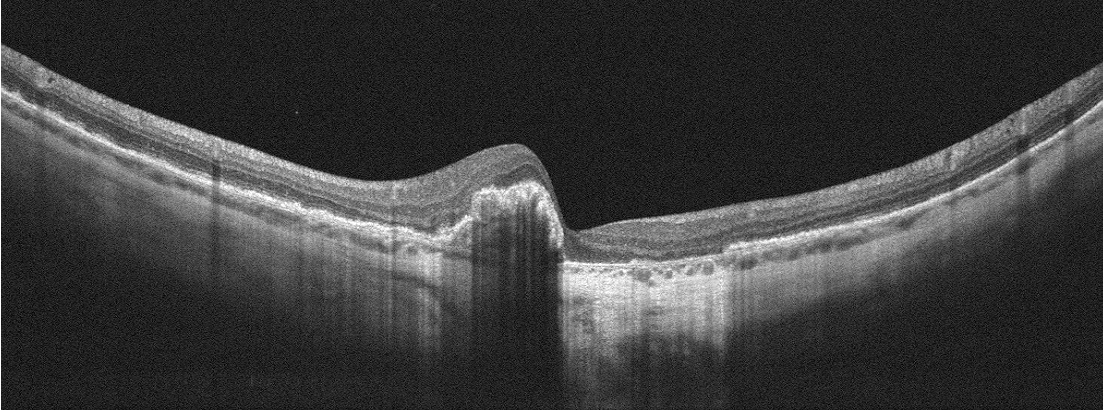

Instrument: Optovue Avanti RTVue XR, optical coherence tomography B-scan — Impression: age-related macular degeneration (AMD).